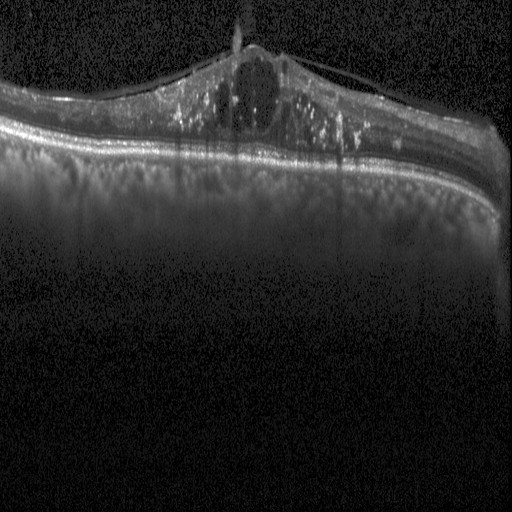

The scan shows diabetic macular edema.